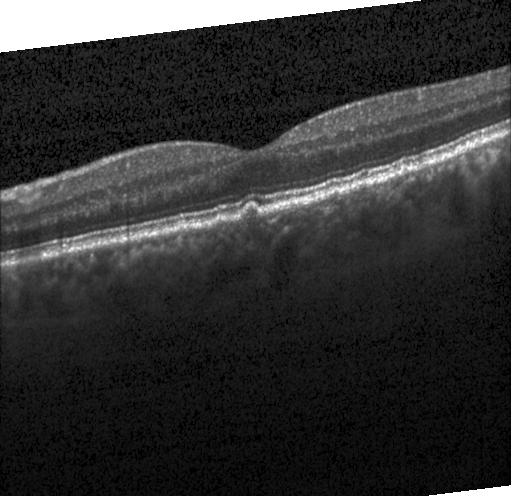

Impression: multiple drusen.